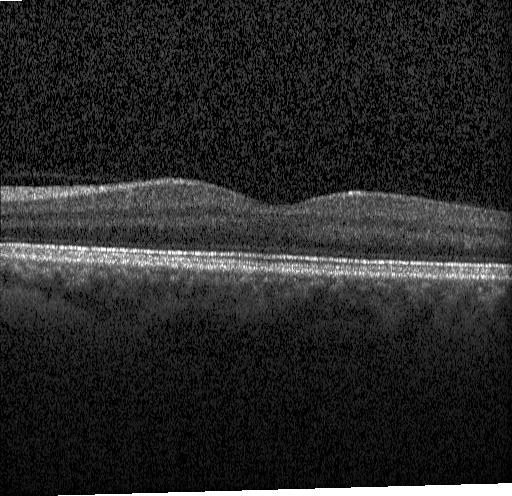
OCT B-scan. The scan shows no choroidal neovascularization, diabetic macular edema, or drusen.